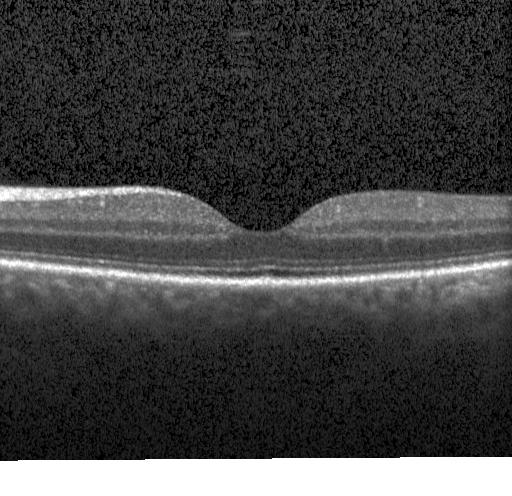
Diagnosis: no choroidal neovascularization, no diabetic macular edema, and no drusen.